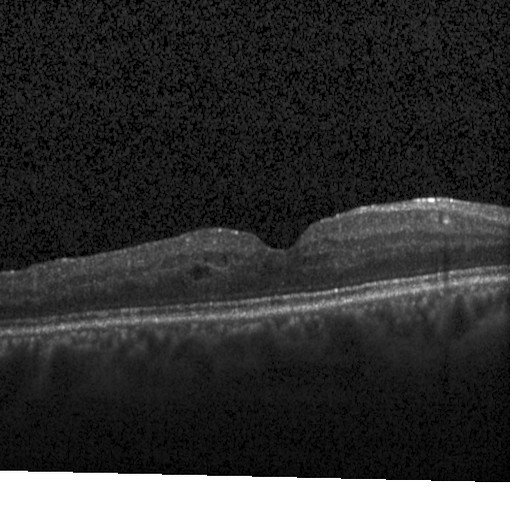
OCT line scan, horizontal scan through the fovea.
Finding: DME.